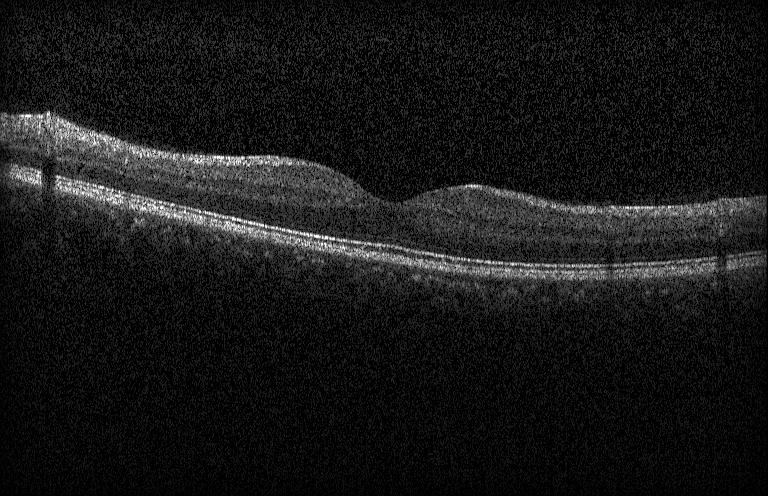 OCT finding: no choroidal neovascularization, diabetic macular edema, or drusen.